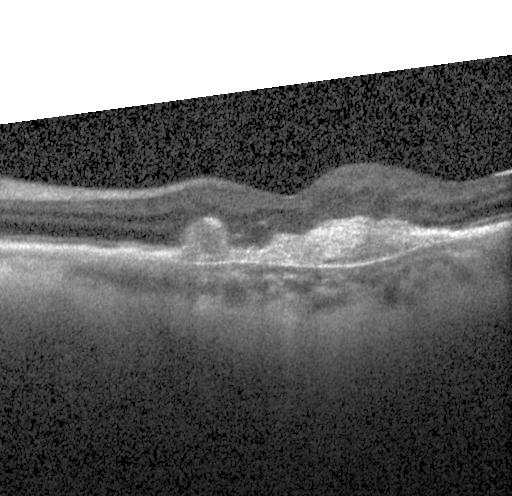 Retinal OCT B-scan — Macular OCT: choroidal neovascularization.